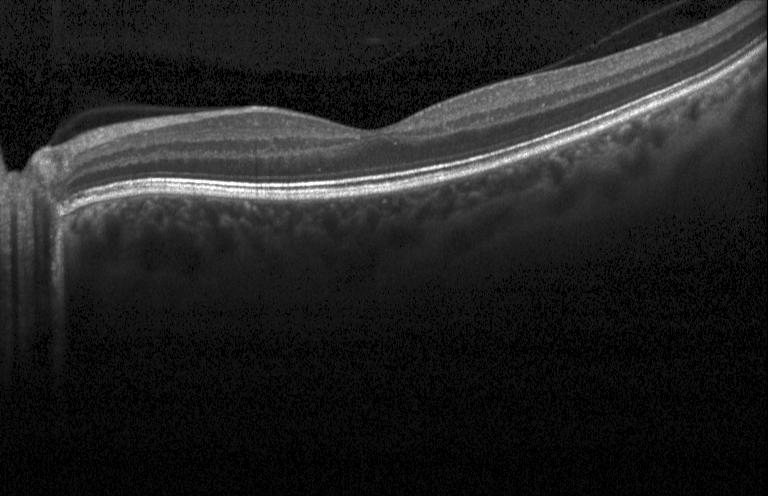

Diagnosis: no evidence of choroidal neovascularization, diabetic macular edema, or drusen.